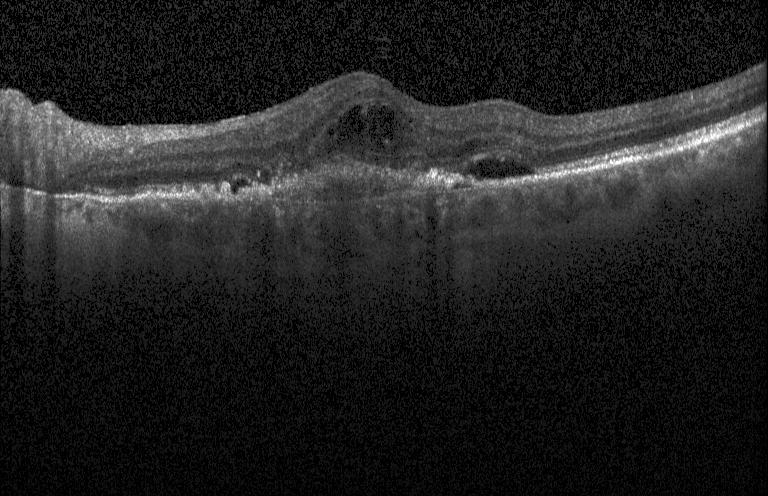 Optical coherence tomography B-scan. Spectral-domain OCT. Acquired on a Heidelberg Spectralis. Centered on the fovea. OCT finding: a choroidal neovascular membrane.